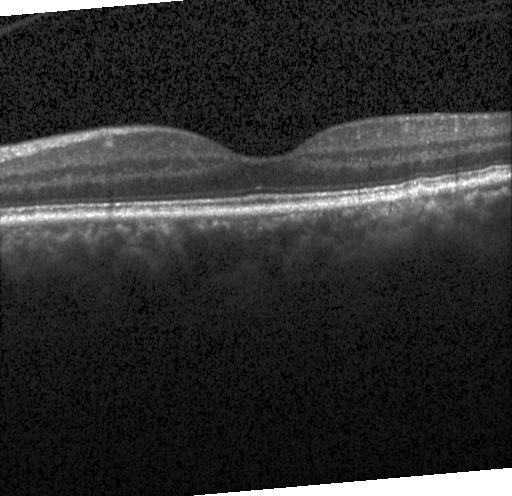
Macular OCT demonstrating neither CNV, DME, nor drusen.